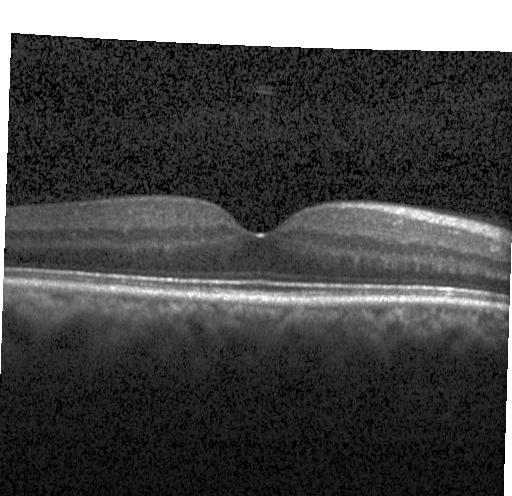
OCT B-scan · Heidelberg Spectralis OCT system · spectral-domain optical coherence tomography. No choroidal neovascularization, no diabetic macular edema, and no drusen.